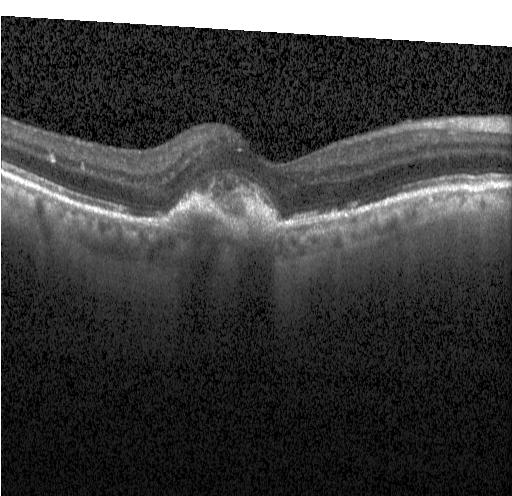 OCT line scan, spectral-domain optical coherence tomography, centered on the fovea. The scan shows a choroidal neovascular membrane.